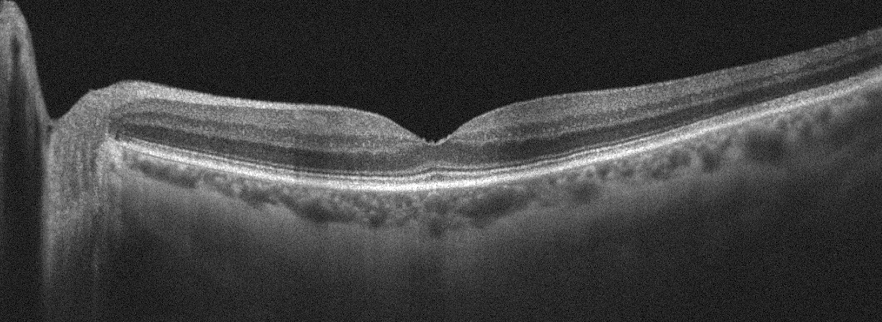

OS; retinal OCT B-scan.
Finding: absence of AMD, DME, ERM, RAO, RVO, and vitreomacular interface disease.